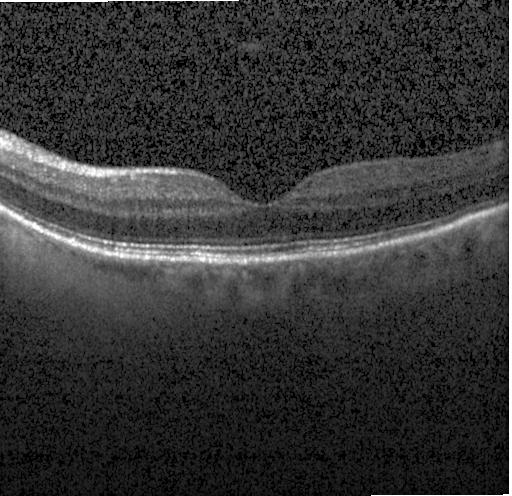

OCT finding: no evidence of choroidal neovascularization, diabetic macular edema, or drusen.